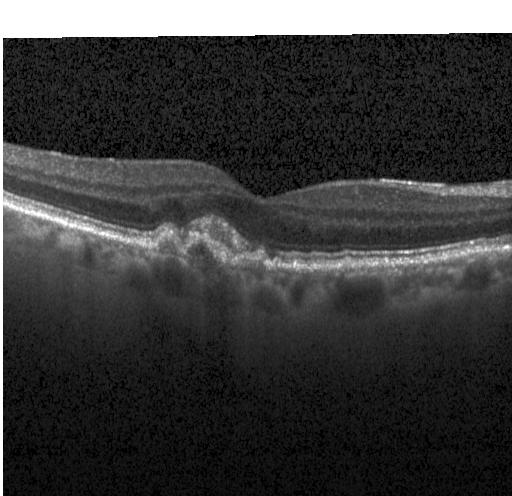
The scan shows CNV.